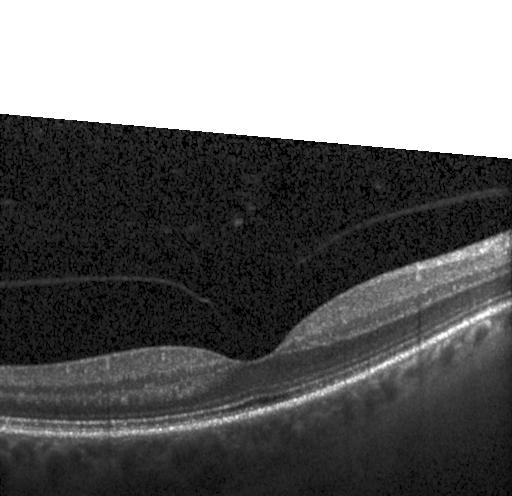

Heidelberg Spectralis. Optical coherence tomography B-scan.
Finding: no evidence of choroidal neovascularization, diabetic macular edema, or drusen.